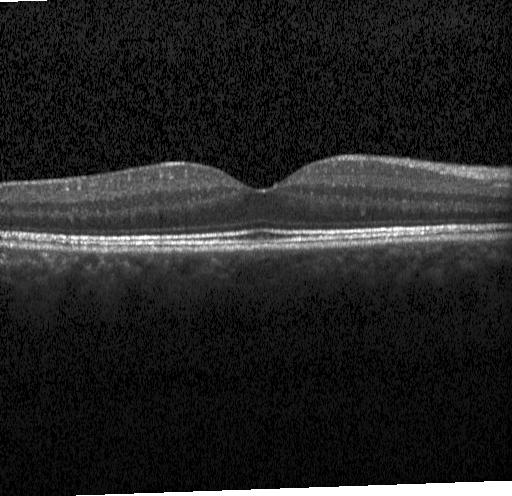
Heidelberg Spectralis OCT system. Optical coherence tomography scan. Diagnosis: neither choroidal neovascularization, diabetic macular edema, nor drusen.